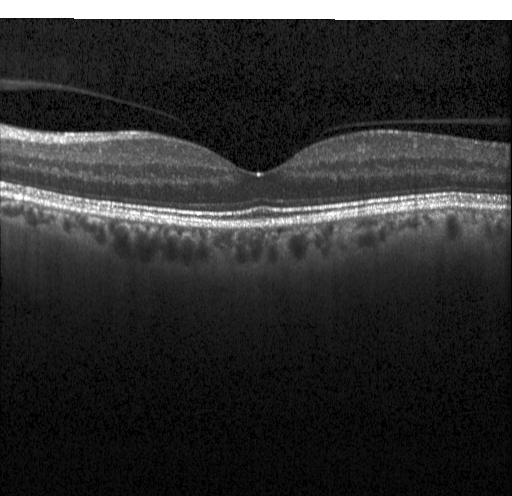
Optical coherence tomography scan.
Diagnosis: no evidence of choroidal neovascularization, diabetic macular edema, or drusen.